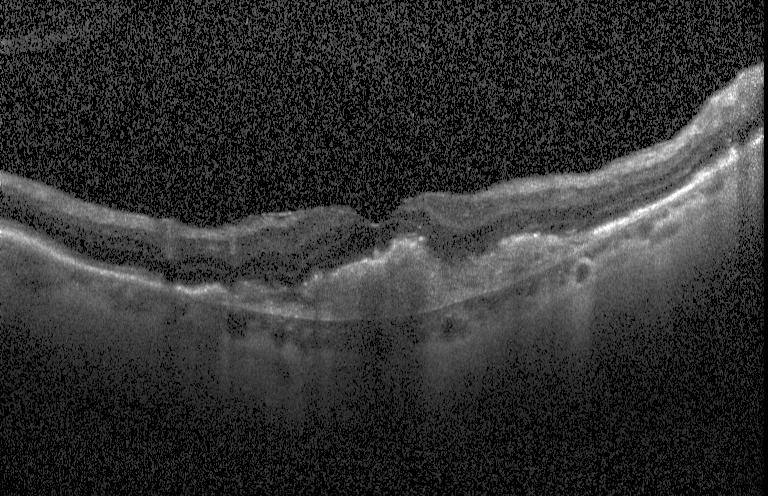

Acquired on a Heidelberg Spectralis, spectral-domain OCT, OCT line scan
Diagnosis: a choroidal neovascular membrane.